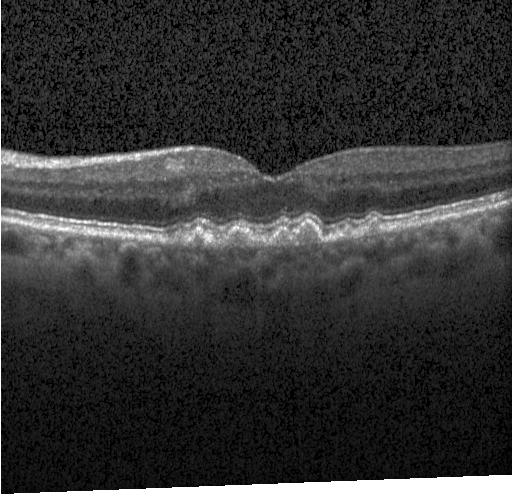

OCT B-scan, spectral-domain optical coherence tomography — Impression: sub-RPE drusenoid deposits.